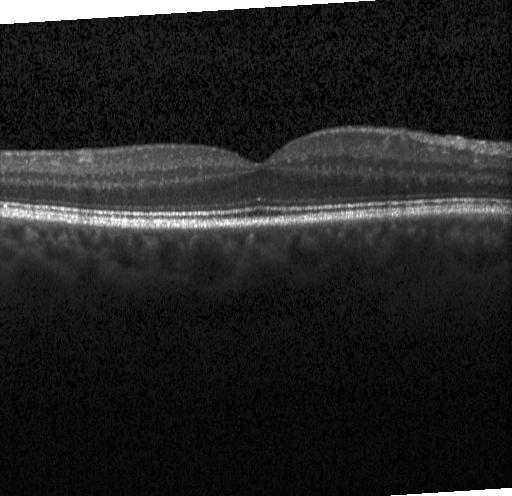

Heidelberg Spectralis; optical coherence tomography scan — This B-scan demonstrates neither choroidal neovascularization, diabetic macular edema, nor drusen.